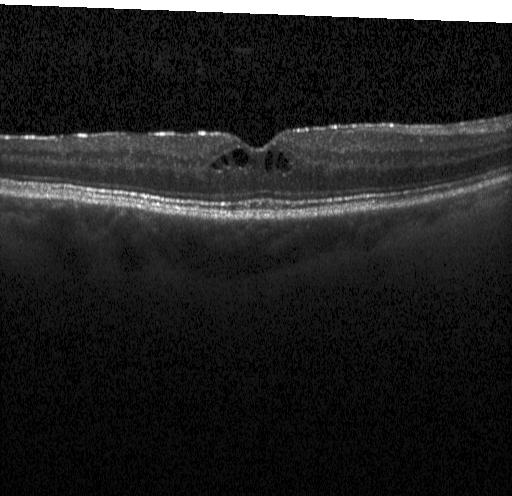 OCT scan showing DME.